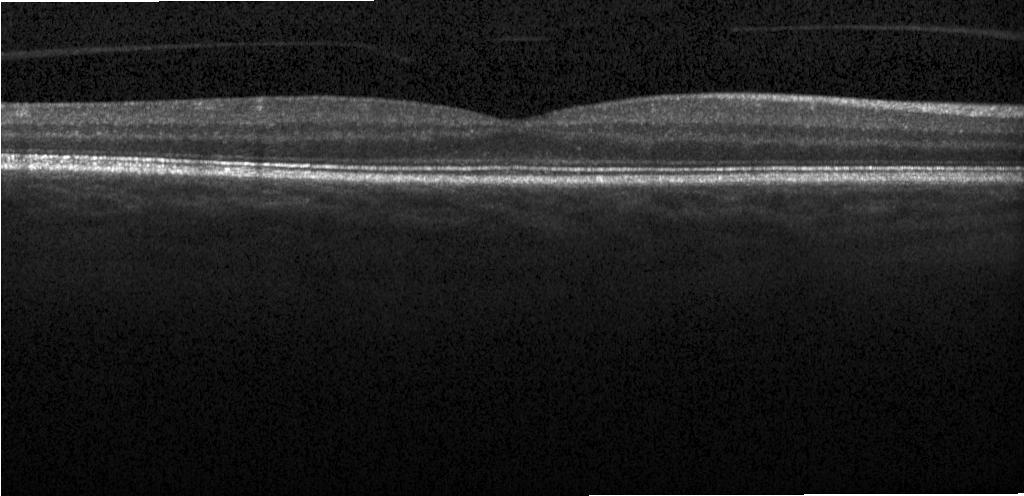 The scan shows neither CNV, DME, nor drusen.